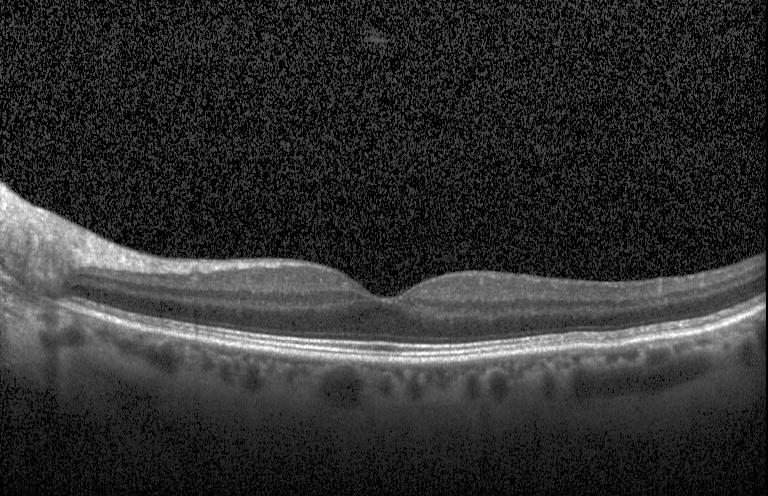

Macular OCT: no evidence of choroidal neovascularization, diabetic macular edema, or drusen.